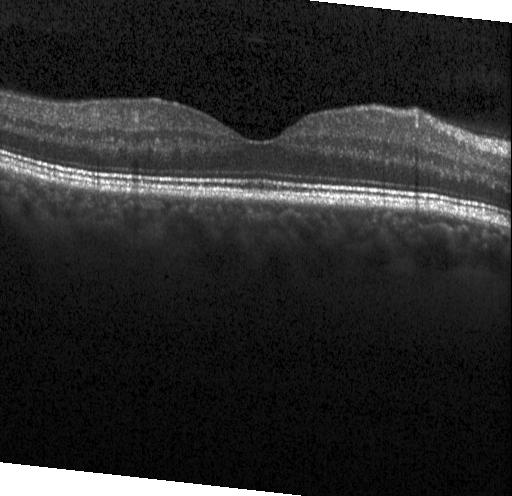

Centered on the fovea, SD-OCT, OCT line scan.
Impression: no choroidal neovascularization, diabetic macular edema, or drusen.